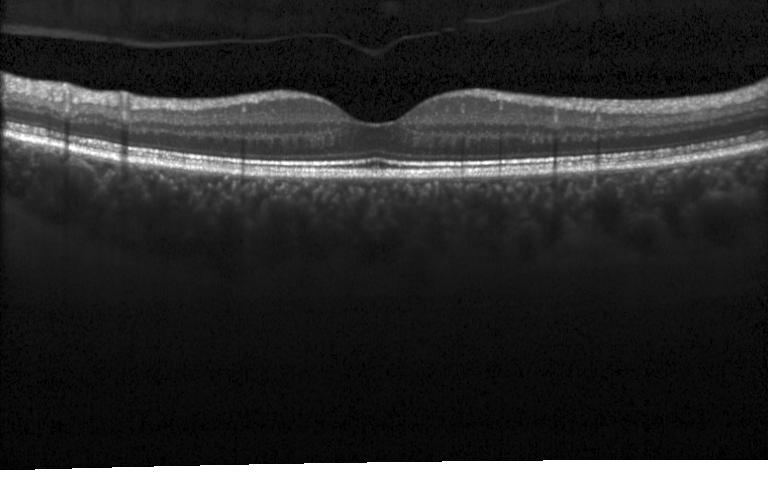

Retinal OCT cross-section showing neither CNV, DME, nor drusen.